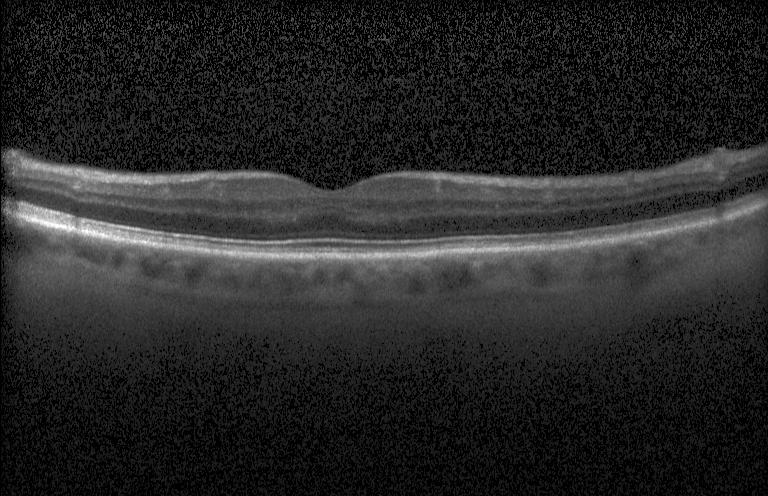
OCT line scan.
The scan shows no evidence of choroidal neovascularization, diabetic macular edema, or drusen.